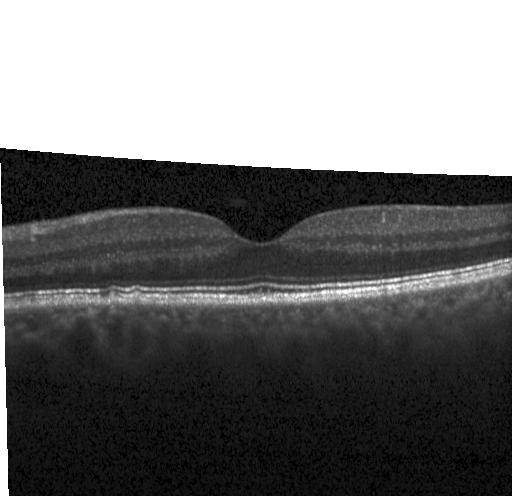

OCT B-scan showing no evidence of choroidal neovascularization, diabetic macular edema, or drusen.